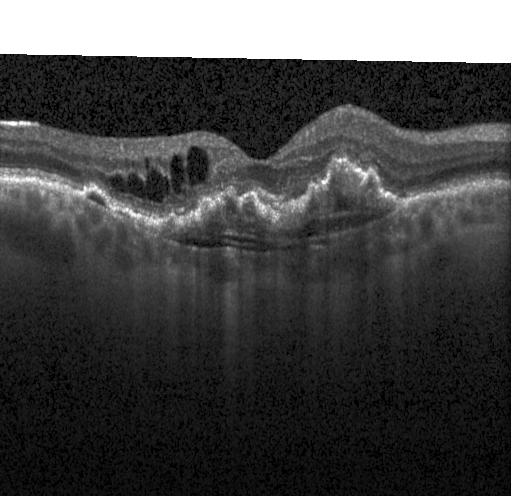 OCT scan showing CNV.